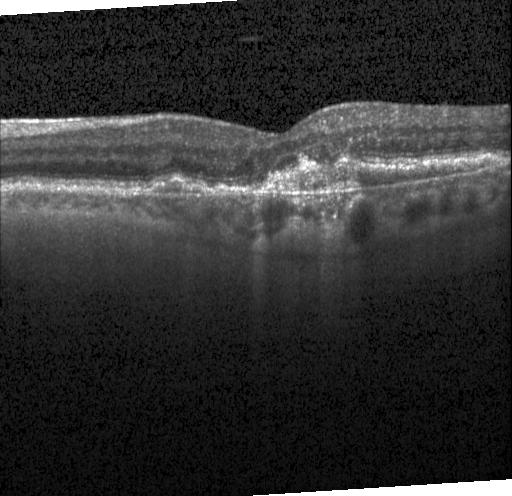 Heidelberg Spectralis OCT system; optical coherence tomography scan. Dx: choroidal neovascularization.